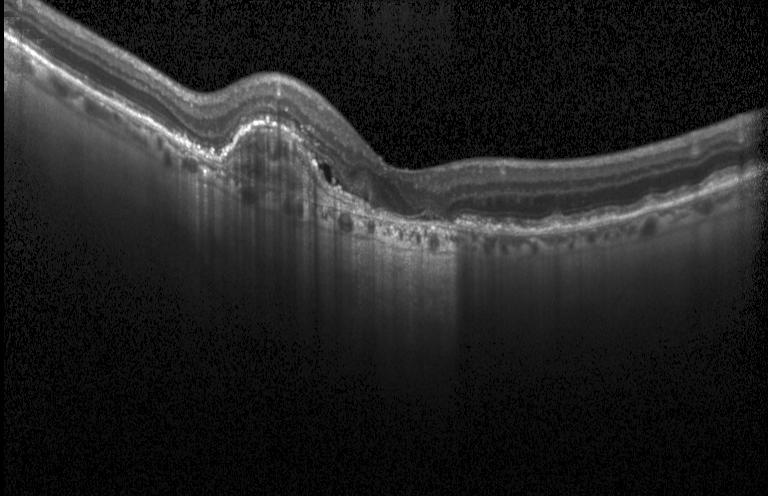 OCT line scan
A choroidal neovascular membrane.